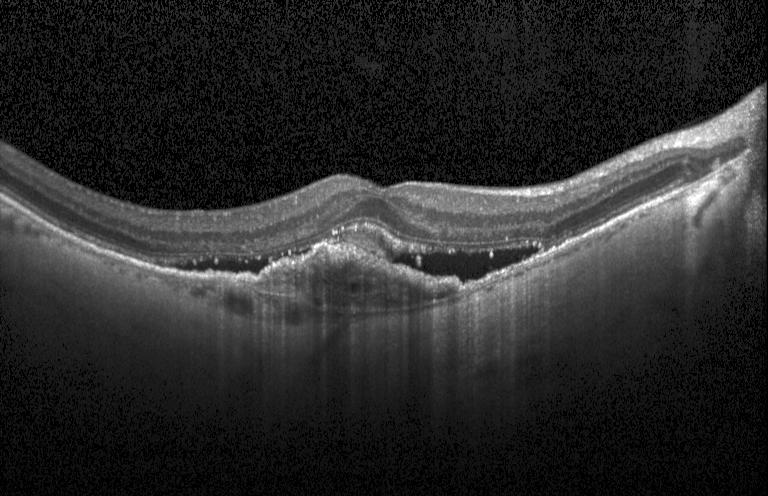 Impression: a choroidal neovascular membrane.